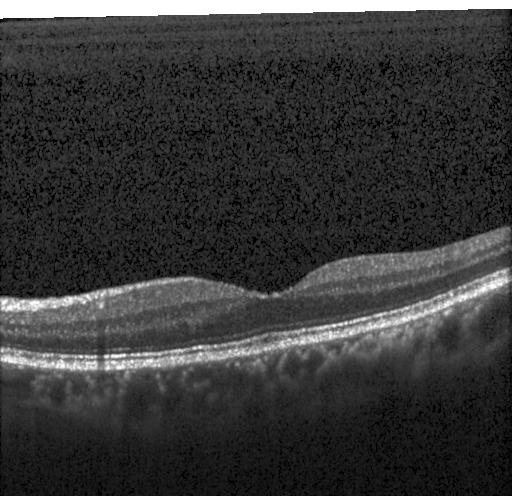
Macular OCT: neither choroidal neovascularization, diabetic macular edema, nor drusen.